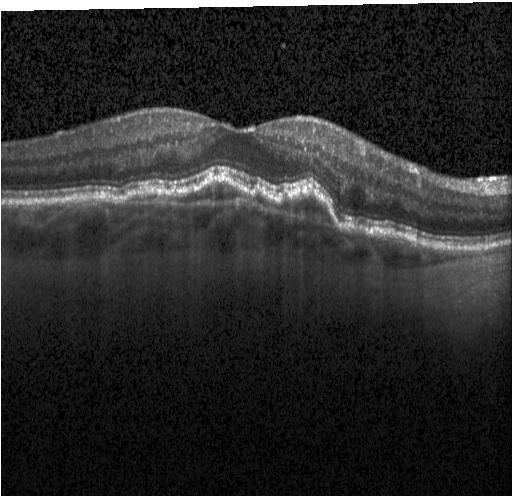 Finding: a choroidal neovascular membrane.